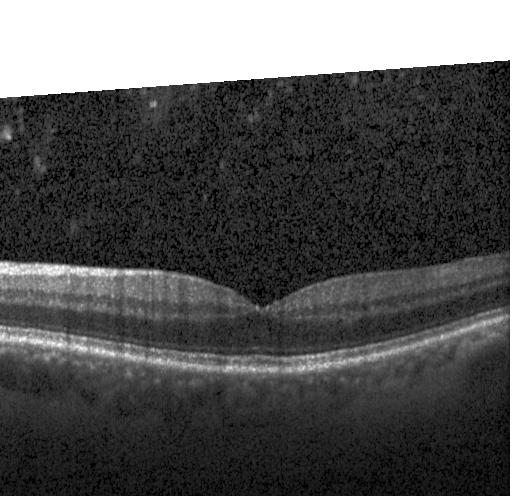
Fovea-centered; retinal OCT B-scan; instrument: Heidelberg Spectralis.
The scan shows no evidence of choroidal neovascularization, diabetic macular edema, or drusen.